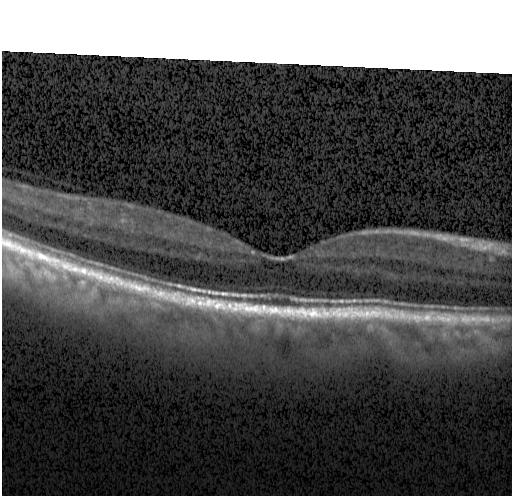
OCT B-scan showing no choroidal neovascularization, diabetic macular edema, or drusen.